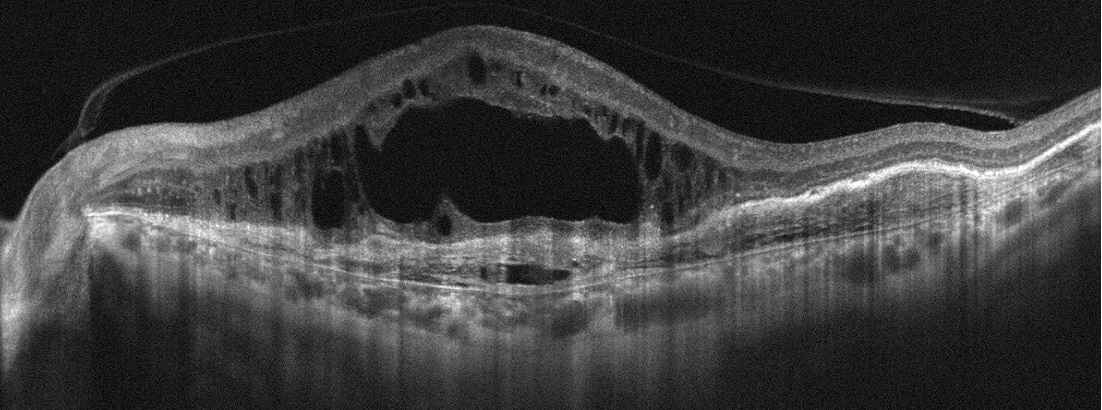

Age-related macular degeneration.